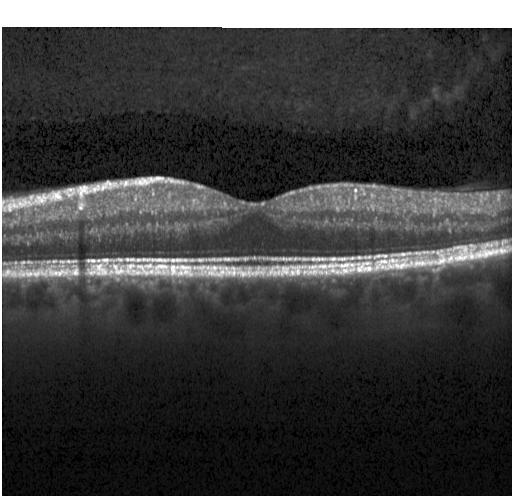

Heidelberg Spectralis, optical coherence tomography scan.
This B-scan demonstrates neither CNV, DME, nor drusen.